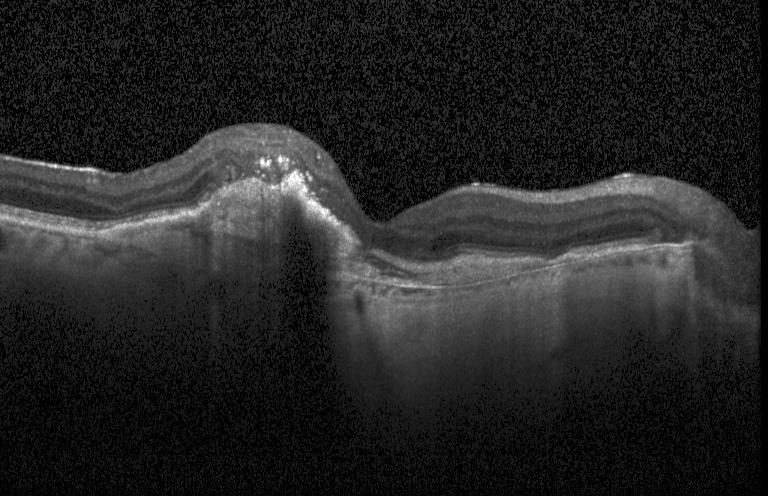 OCT line scan; horizontal scan through the fovea; spectral-domain OCT.
Macular OCT: CNV.